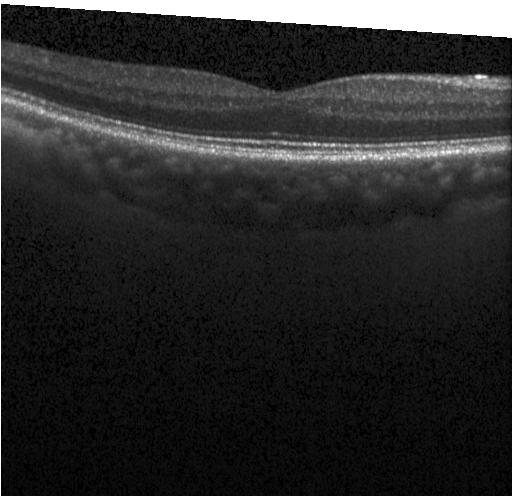 Spectral-domain OCT, retinal OCT cross-section, macular scan — OCT finding: no choroidal neovascularization, no diabetic macular edema, and no drusen.